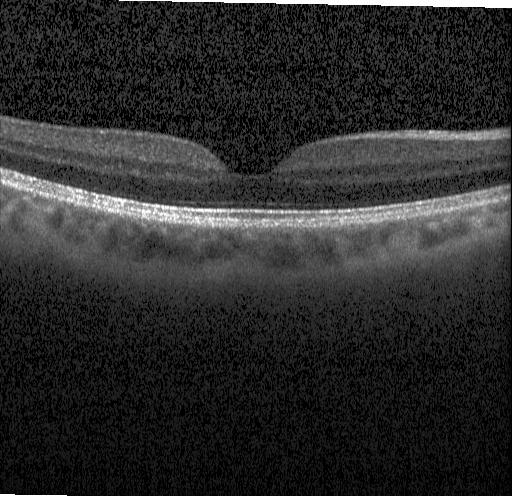 Assessment: no CNV, DME, or drusen.